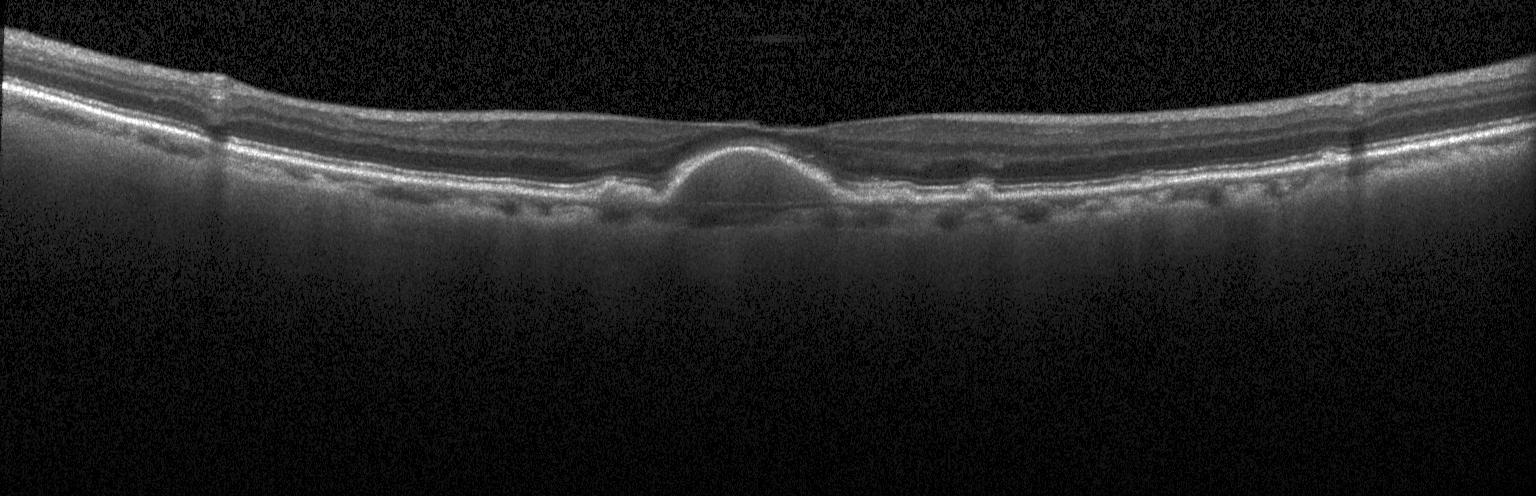
OCT line scan
Diagnosis: a choroidal neovascular membrane.